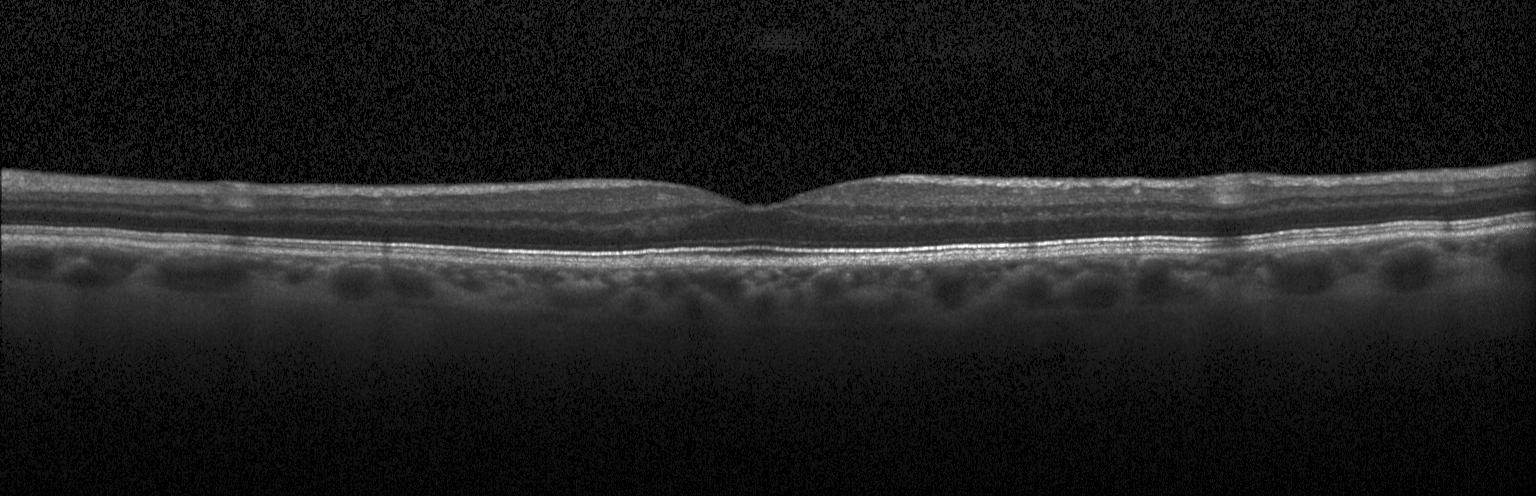

Diagnosis: no CNV, DME, or drusen.